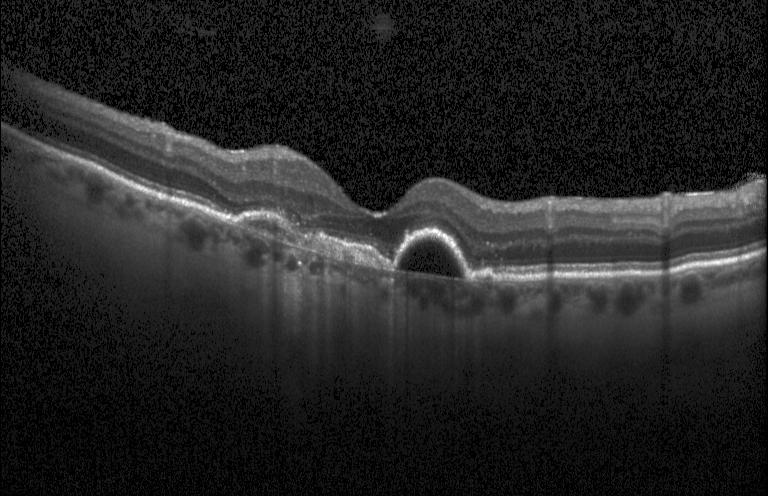 Macular scan; instrument: Heidelberg Spectralis; spectral-domain optical coherence tomography; retinal OCT cross-section
Dx: CNV.